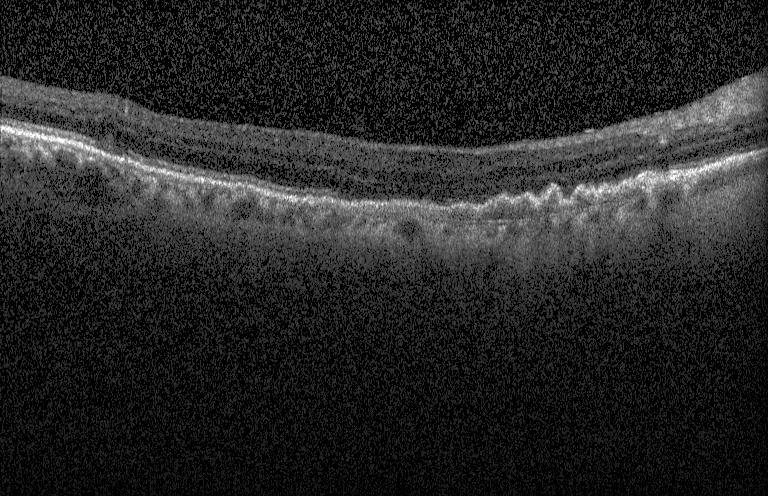 Retinal OCT B-scan, spectral-domain OCT, macular scan — Macular OCT: choroidal neovascularization.